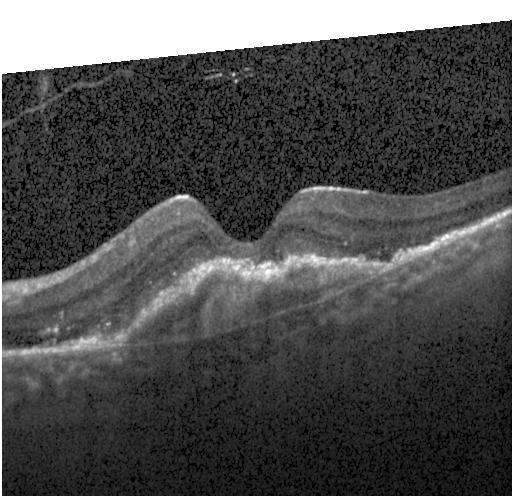 Optical coherence tomography B-scan. OCT finding: a choroidal neovascular membrane.